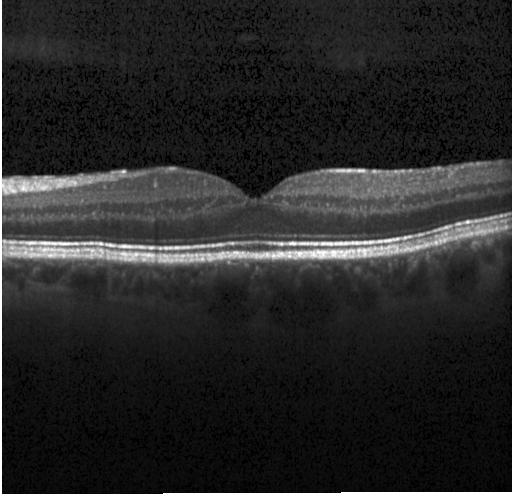

Centered on the fovea. Heidelberg Spectralis. Spectral-domain OCT. Optical coherence tomography scan.
Macular OCT: no CNV, DME, or drusen.